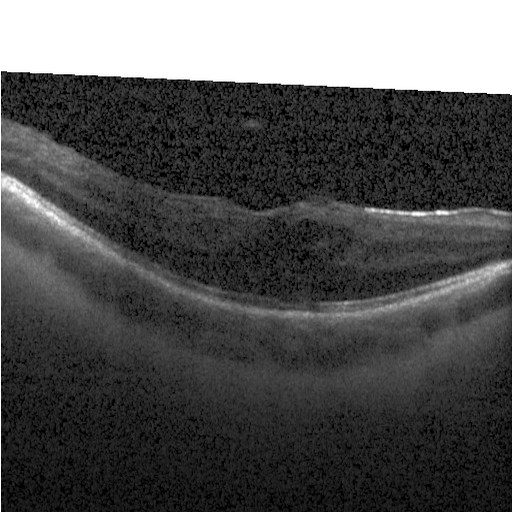

Diagnosis: diabetic macular edema.